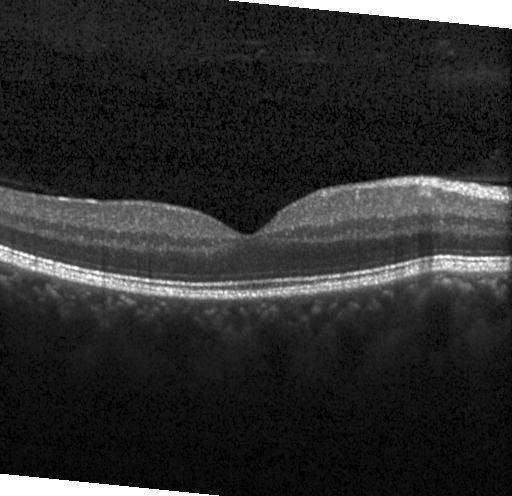
OCT B-scan.
Dx: no evidence of choroidal neovascularization, diabetic macular edema, or drusen.